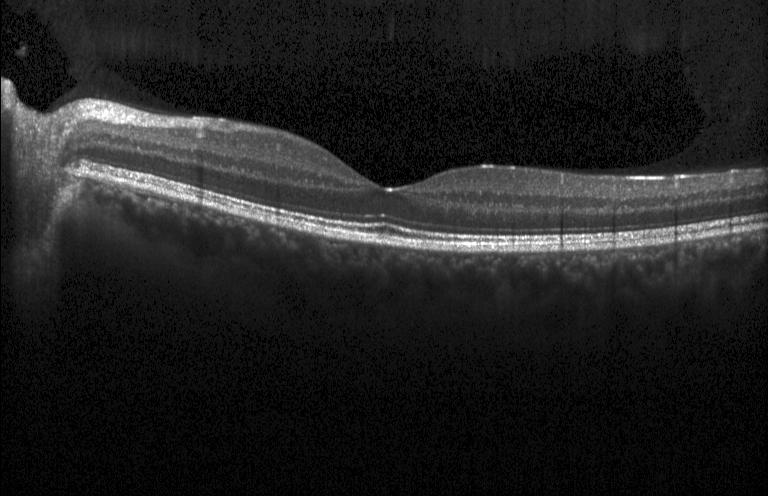 Finding: no CNV, no DME, and no drusen.